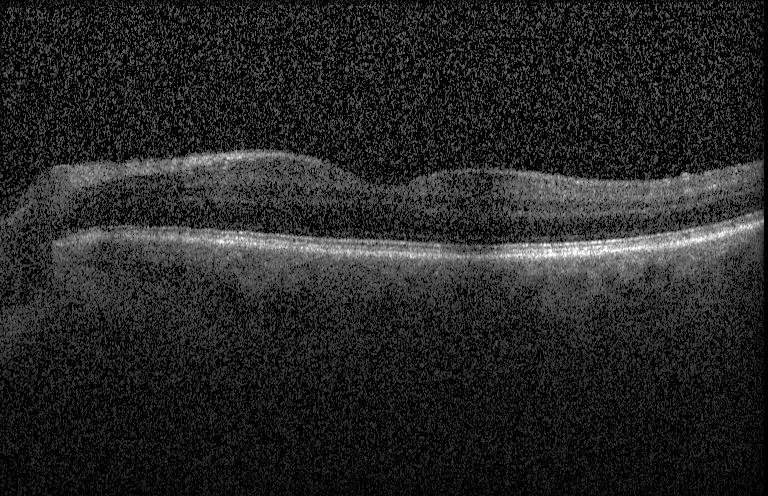 OCT finding: no choroidal neovascularization, diabetic macular edema, or drusen.